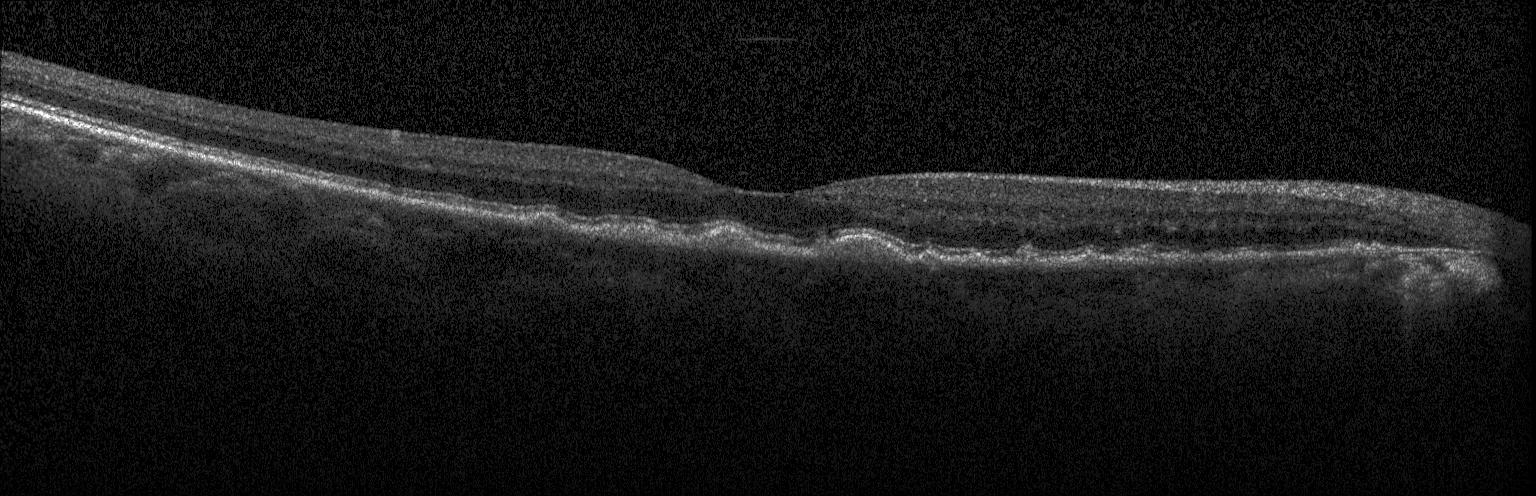
Macular OCT demonstrating drusen.